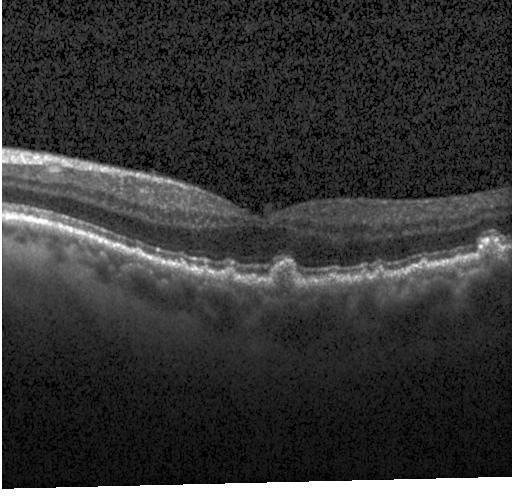 Through the macula, OCT B-scan — The scan shows multiple drusen.